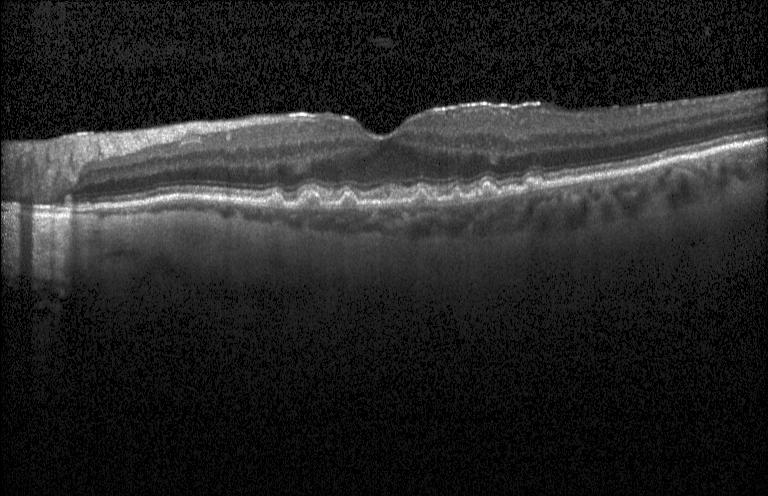 Heidelberg Spectralis OCT system, retinal OCT cross-section.
OCT finding: sub-RPE drusenoid deposits.